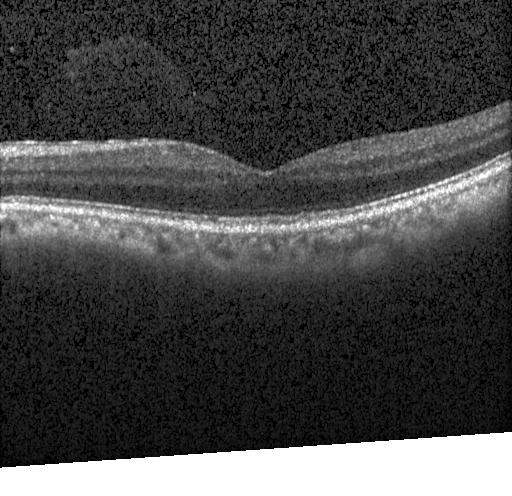
Assessment: no CNV, no DME, and no drusen.